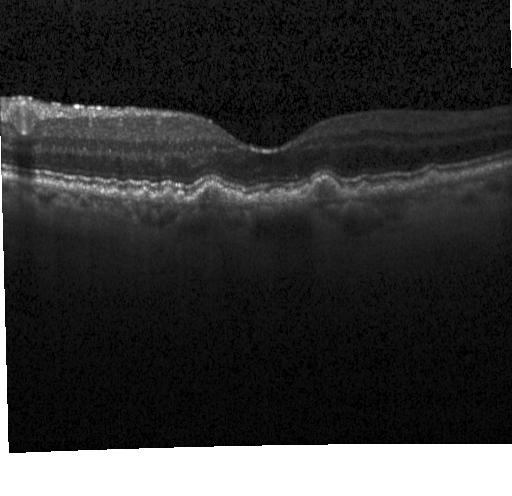

OCT B-scan showing sub-RPE drusenoid deposits.